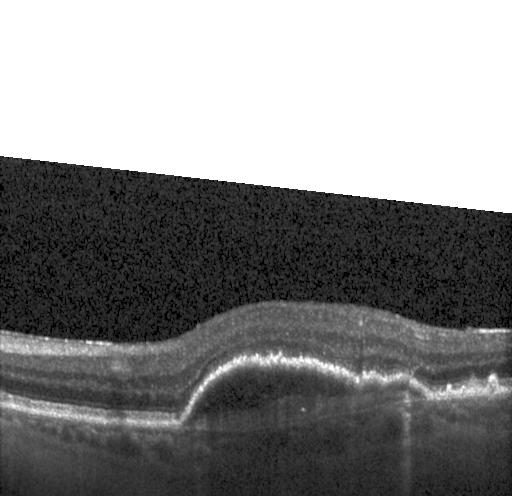 Retinal OCT B-scan, SD-OCT.
The scan shows CNV.